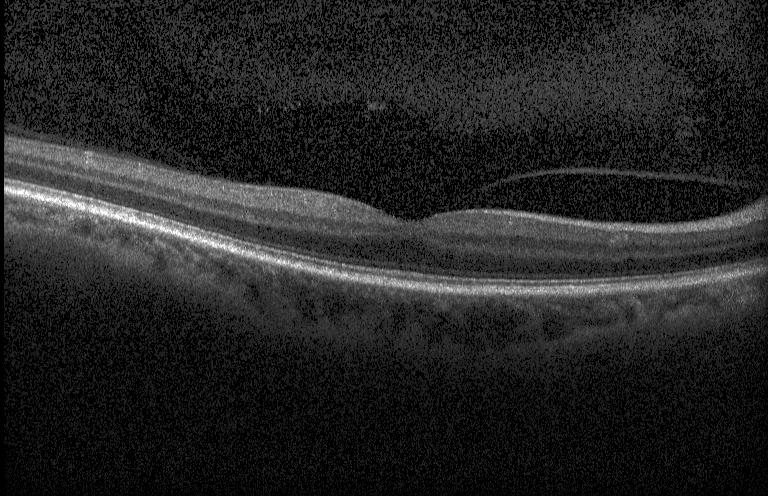
Finding: neither CNV, DME, nor drusen.